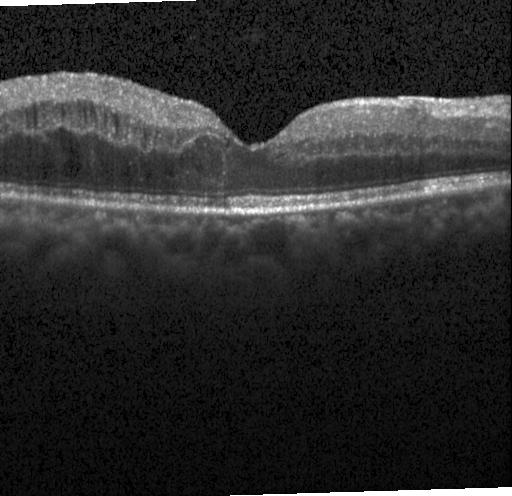
Assessment: diabetic macular edema.